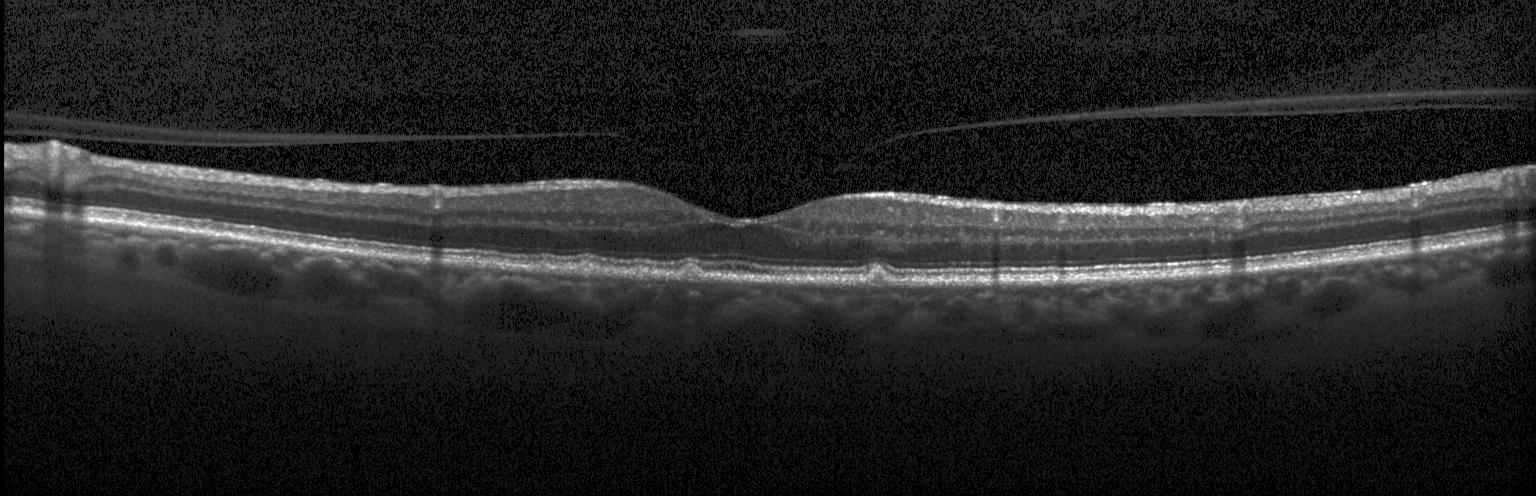 Retinal OCT cross-section, fovea-centered, Heidelberg Spectralis OCT system, spectral-domain OCT
Finding: drusen.